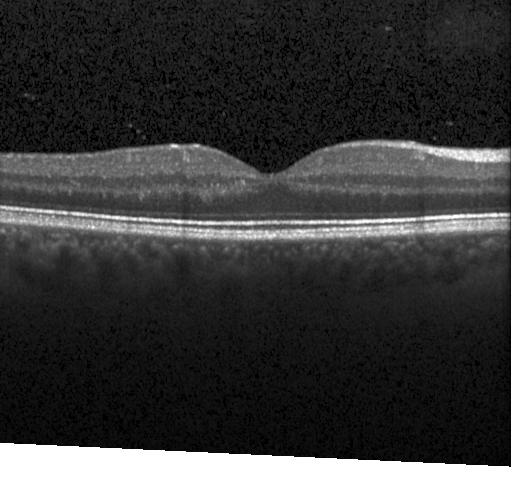

Optical coherence tomography scan
The scan shows no choroidal neovascularization, diabetic macular edema, or drusen.